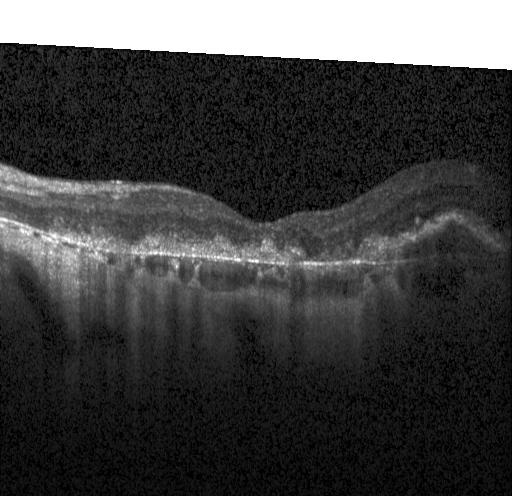

Optical coherence tomography B-scan.
Impression: choroidal neovascularization.